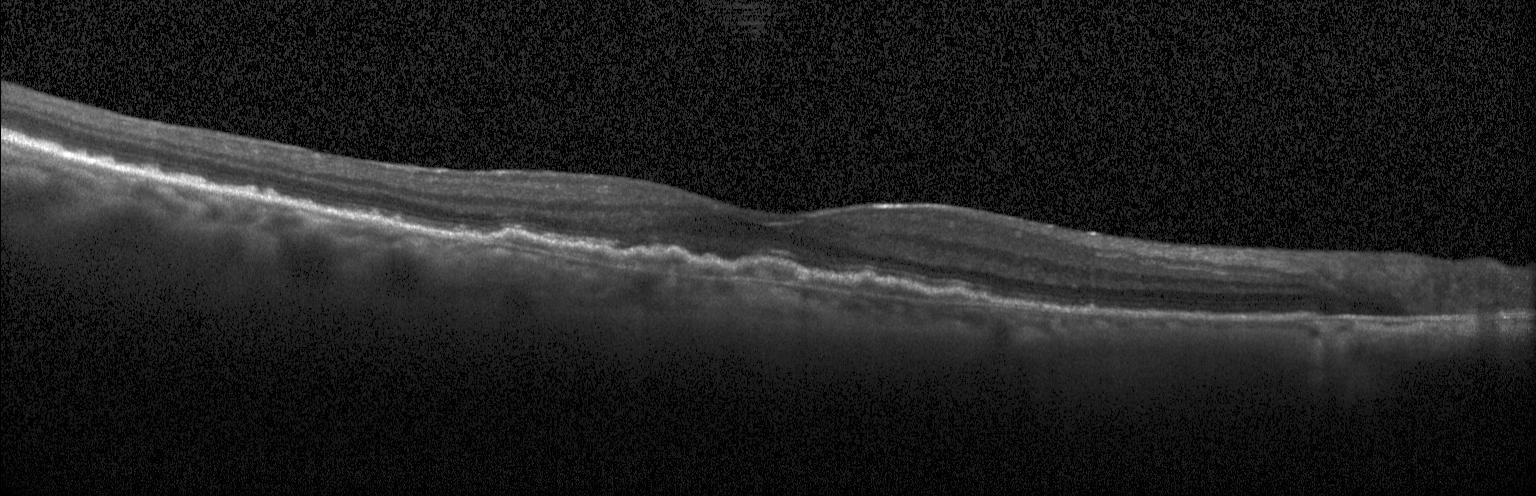 Spectral-domain OCT, optical coherence tomography B-scan, acquired on a Heidelberg Spectralis, through the macula — Impression: CNV.